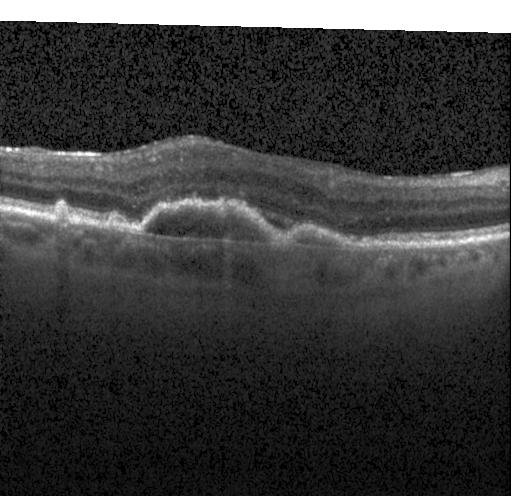
Horizontal scan through the fovea · SD-OCT · Heidelberg Spectralis · retinal OCT B-scan — This B-scan demonstrates a choroidal neovascular membrane.